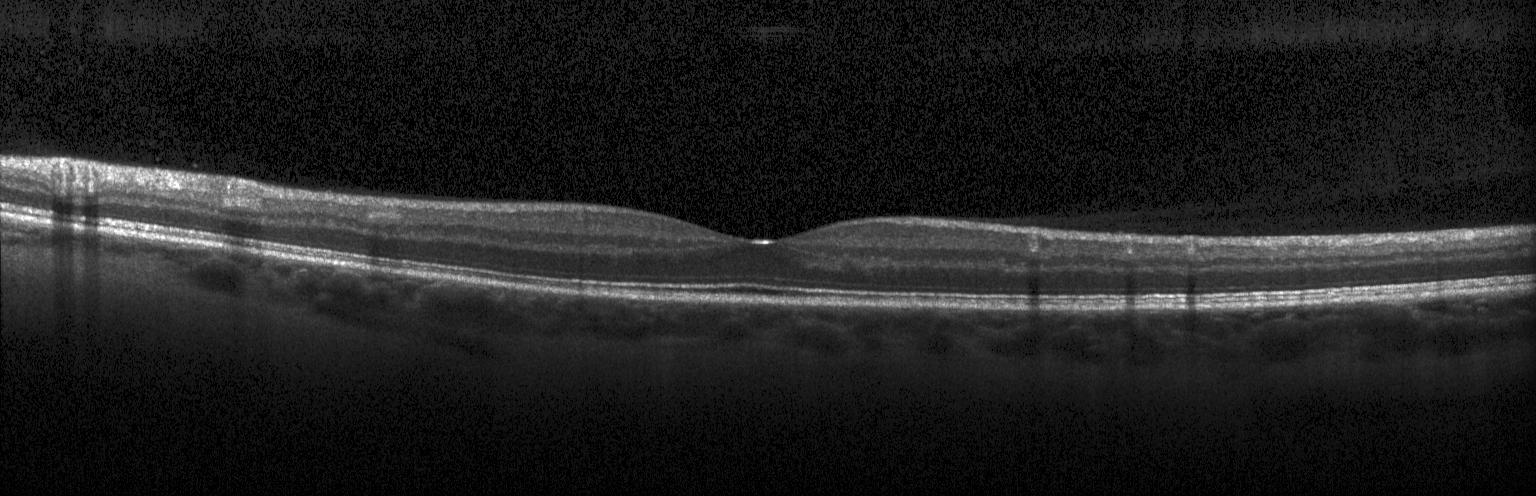

OCT scan showing no choroidal neovascularization, diabetic macular edema, or drusen.